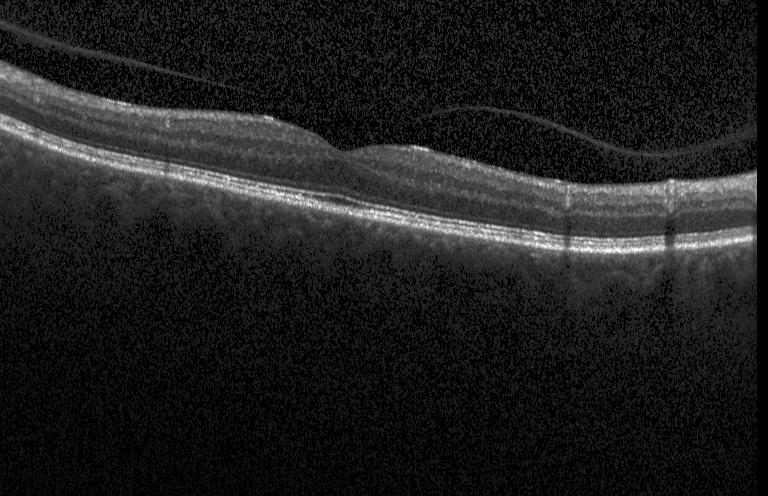

Acquired on a Heidelberg Spectralis; retinal OCT B-scan; fovea-centered.
OCT finding: no choroidal neovascularization, no diabetic macular edema, and no drusen.